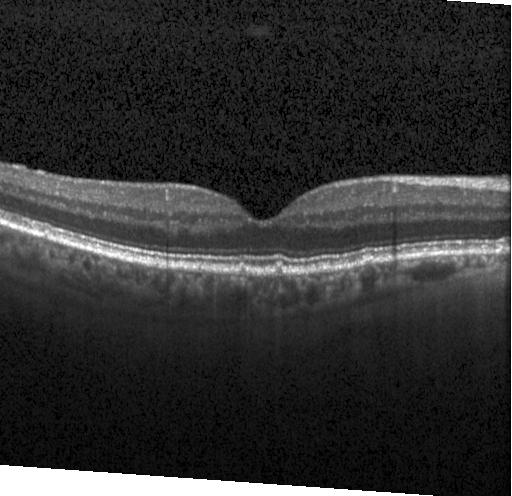 OCT finding: drusen.